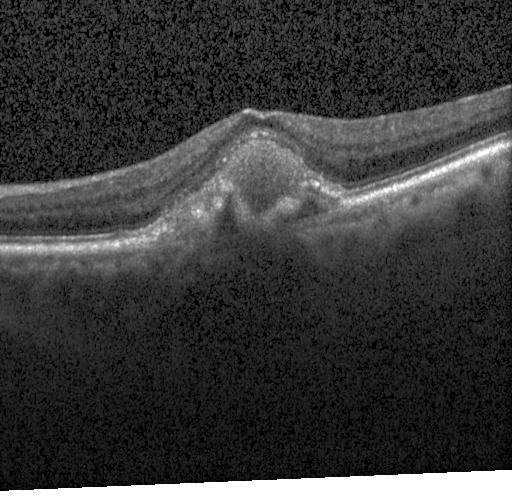
Acquired on a Heidelberg Spectralis; fovea-centered; OCT line scan; SD-OCT.
Impression: a choroidal neovascular membrane.